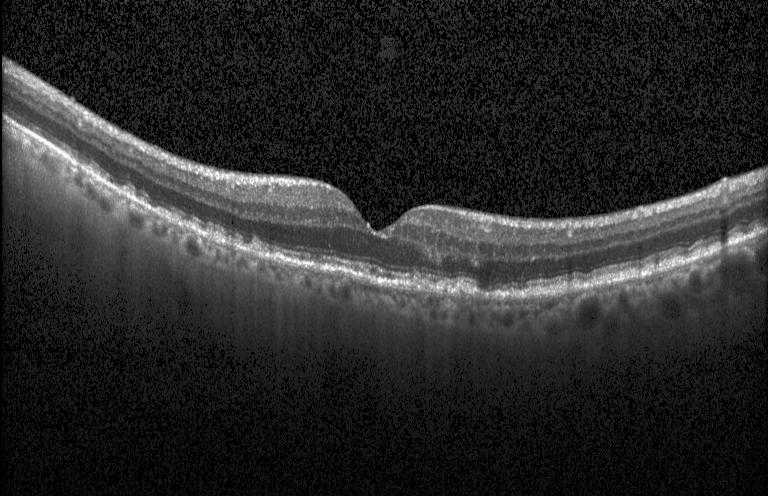
Fovea-centered. Retinal OCT B-scan.
Multiple drusen.